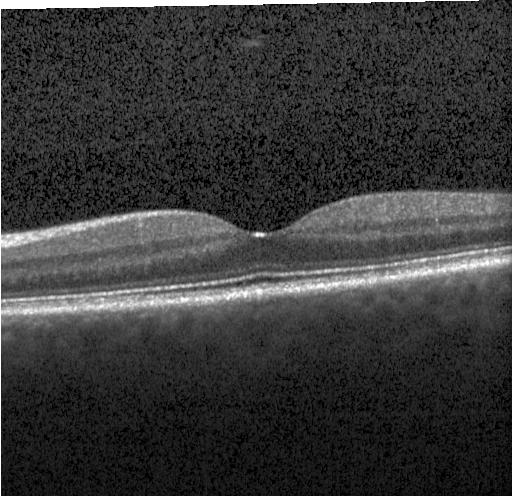 Dx: no evidence of CNV, DME, or drusen.